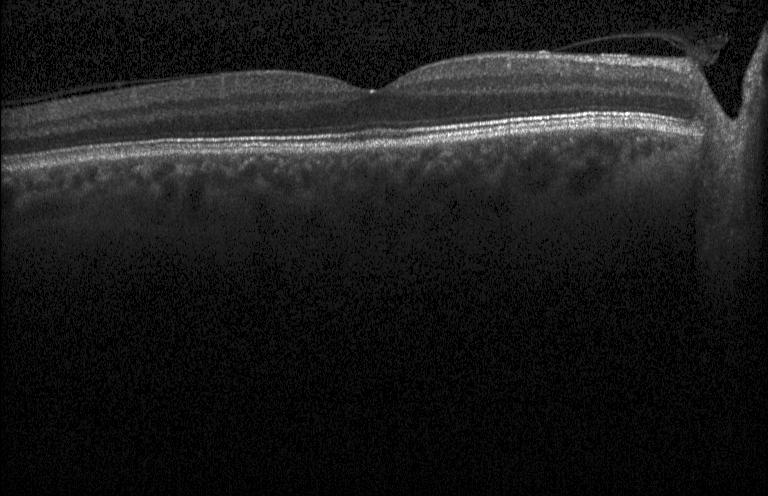
Optical coherence tomography scan; Heidelberg Spectralis; horizontal scan through the fovea
Macular OCT: neither choroidal neovascularization, diabetic macular edema, nor drusen.